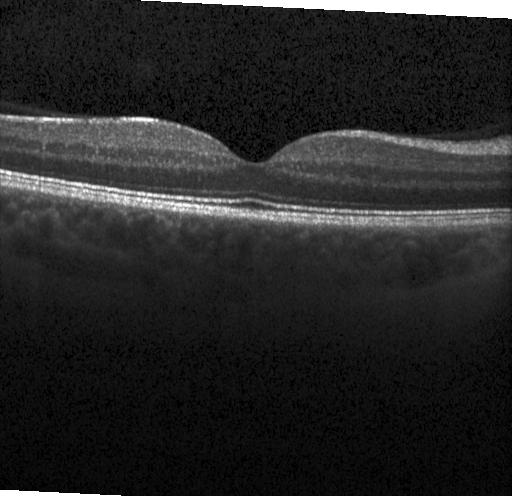
OCT B-scan. Spectral-domain OCT. Through the macula. Heidelberg Spectralis OCT system. Finding: no choroidal neovascularization, no diabetic macular edema, and no drusen.